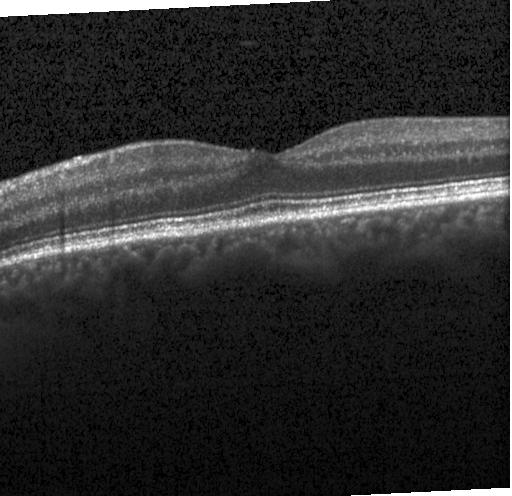

Acquired on a Heidelberg Spectralis, fovea-centered, spectral-domain optical coherence tomography, retinal OCT cross-section
OCT finding: no choroidal neovascularization, diabetic macular edema, or drusen.